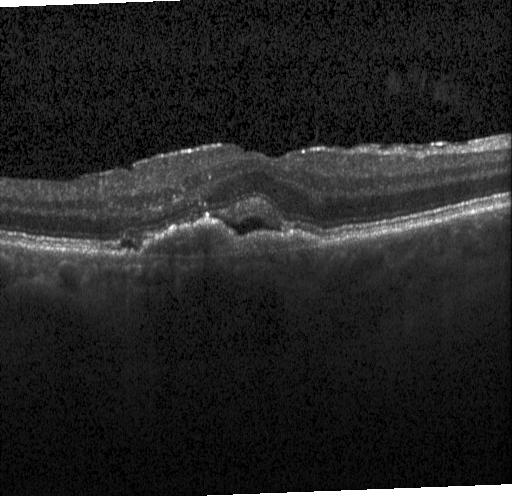 Spectral-domain optical coherence tomography, OCT line scan
The scan shows choroidal neovascularization (CNV).